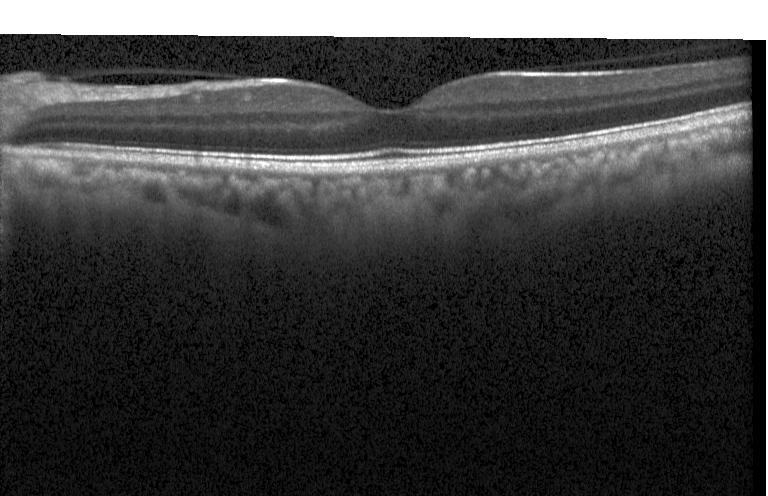 Impression: neither choroidal neovascularization, diabetic macular edema, nor drusen.